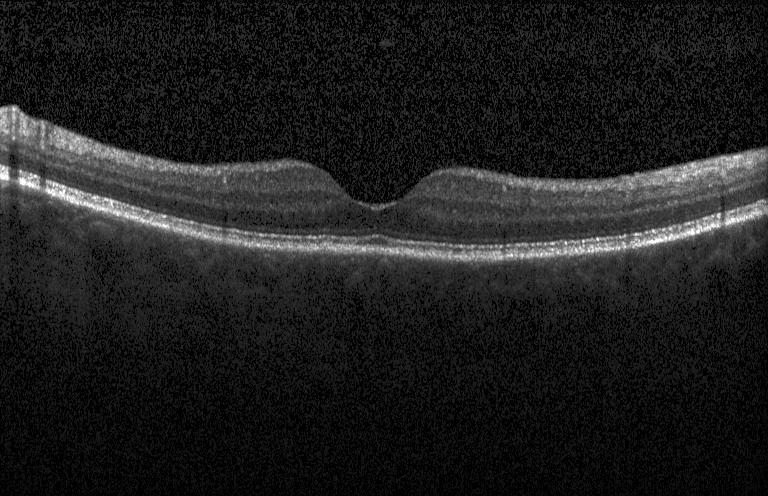

OCT scan showing no evidence of CNV, DME, or drusen.